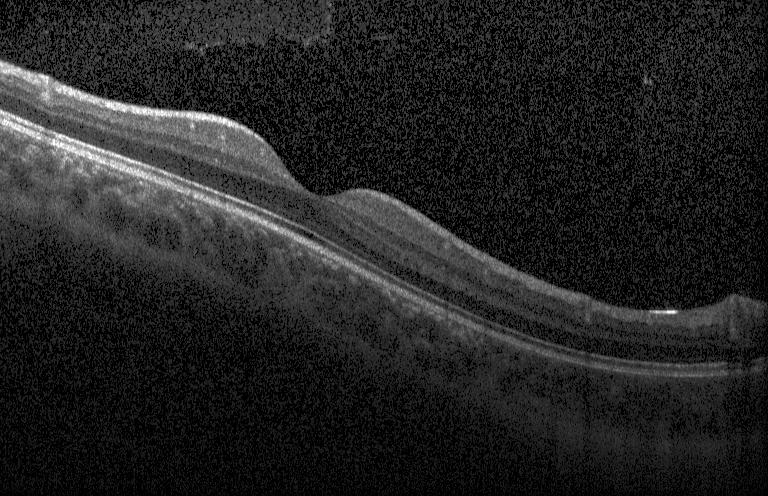
OCT B-scan showing neither choroidal neovascularization, diabetic macular edema, nor drusen.